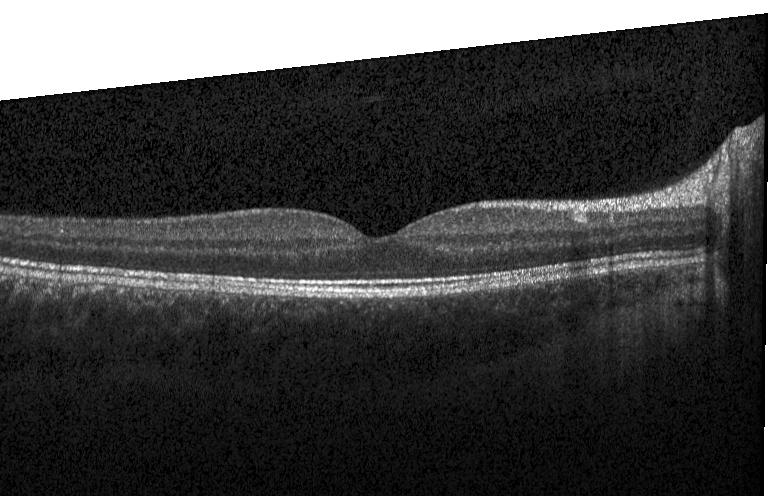

Retinal OCT B-scan. Dx: no evidence of CNV, DME, or drusen.